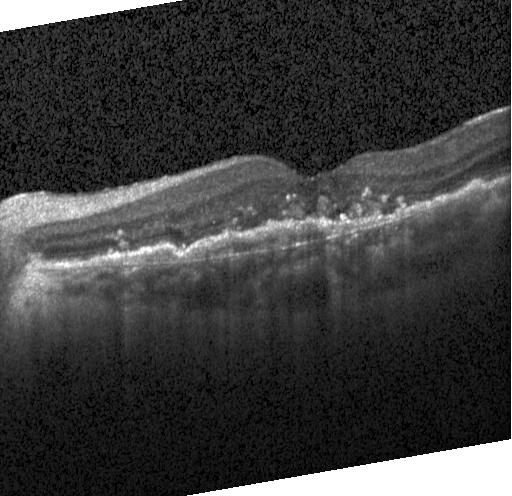 Macular OCT: a choroidal neovascular membrane.